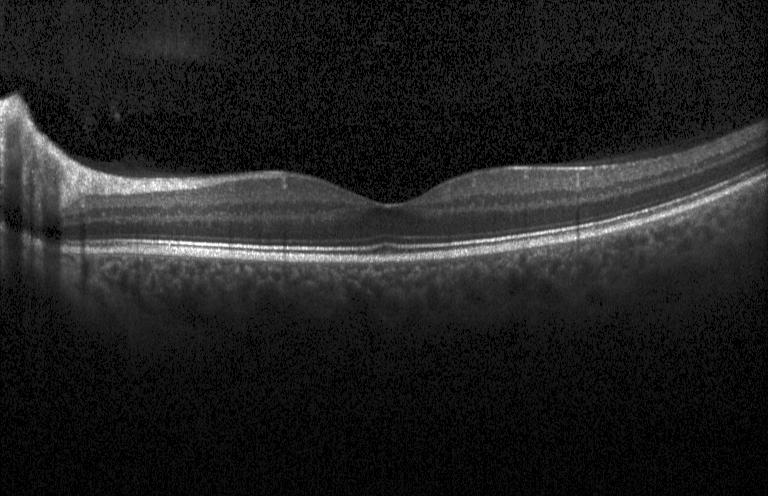

Macular OCT: no choroidal neovascularization, diabetic macular edema, or drusen.